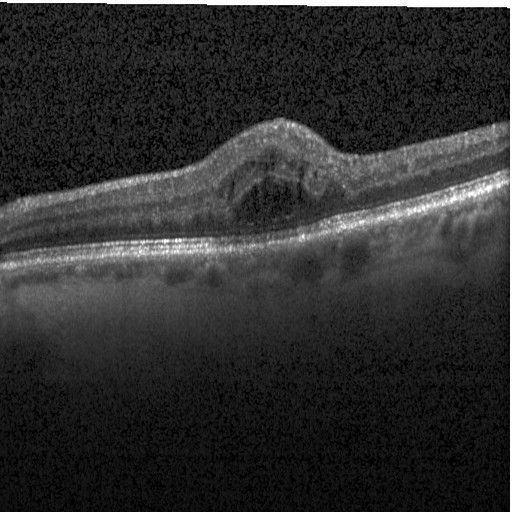 Retinal OCT cross-section; acquired on a Heidelberg Spectralis; horizontal scan through the fovea
Macular OCT: DME.